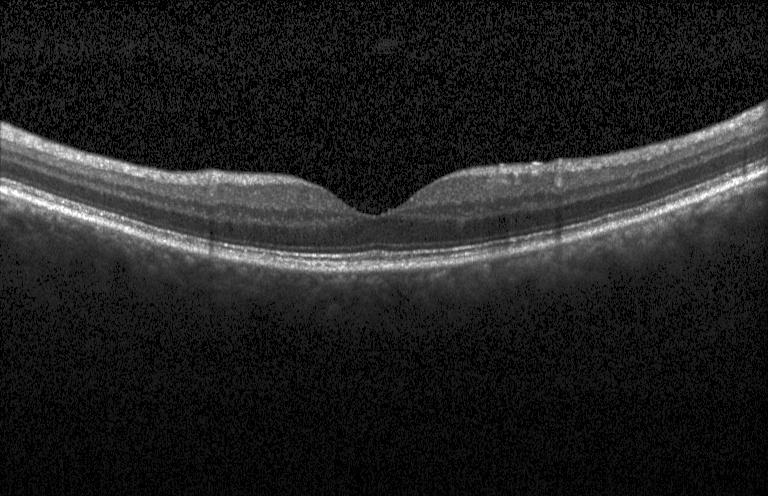
Instrument: Heidelberg Spectralis. Centered on the fovea. Spectral-domain OCT. Optical coherence tomography scan.
Diagnosis: no evidence of choroidal neovascularization, diabetic macular edema, or drusen.